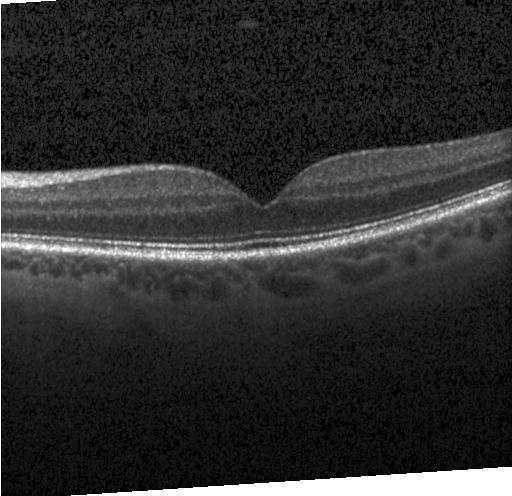

Macular OCT: neither CNV, DME, nor drusen.